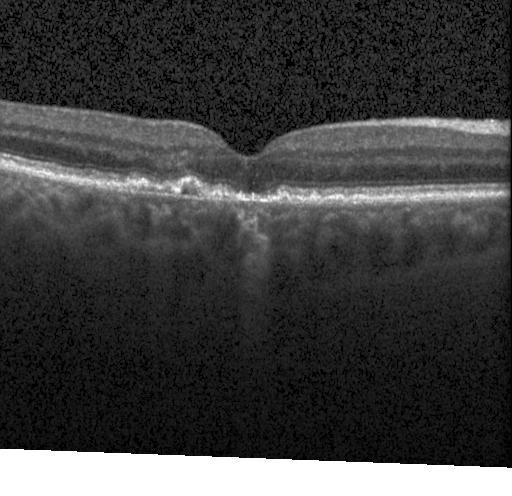

Spectral-domain optical coherence tomography · centered on the fovea · acquired on a Heidelberg Spectralis · optical coherence tomography scan. A choroidal neovascular membrane.